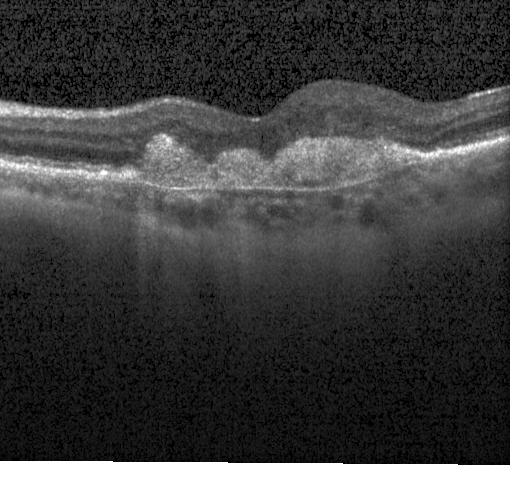
OCT line scan.
Finding: CNV.